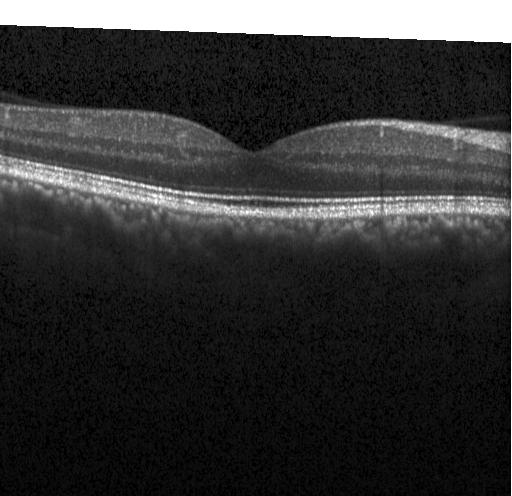

Diagnosis: no choroidal neovascularization, no diabetic macular edema, and no drusen.